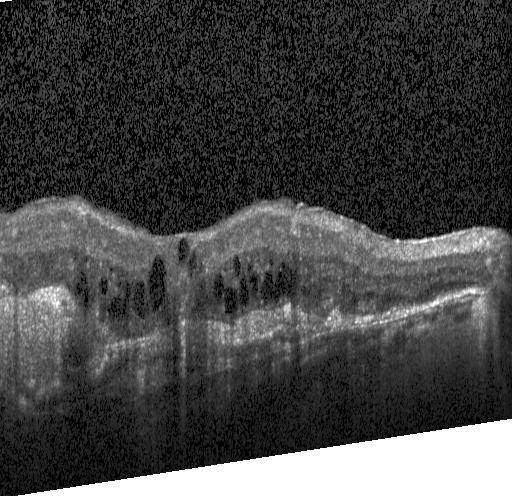

Through the macula · OCT B-scan · acquired on a Heidelberg Spectralis. Impression: choroidal neovascularization (CNV).